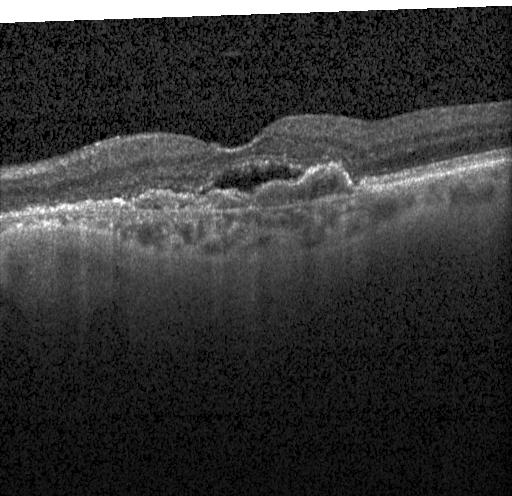

Retinal OCT B-scan, SD-OCT, macular scan, Heidelberg Spectralis
Diagnosis: a choroidal neovascular membrane.